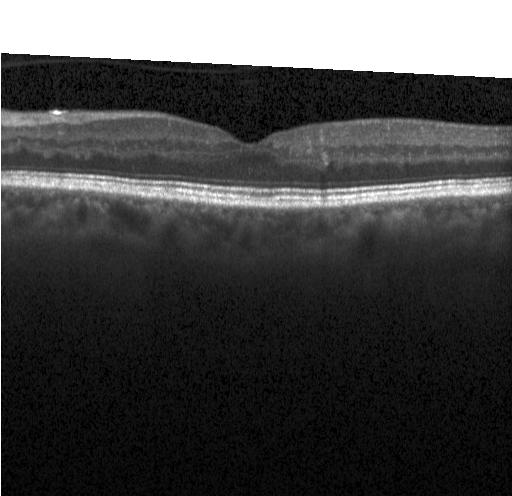

Optical coherence tomography scan. This B-scan demonstrates neither choroidal neovascularization, diabetic macular edema, nor drusen.